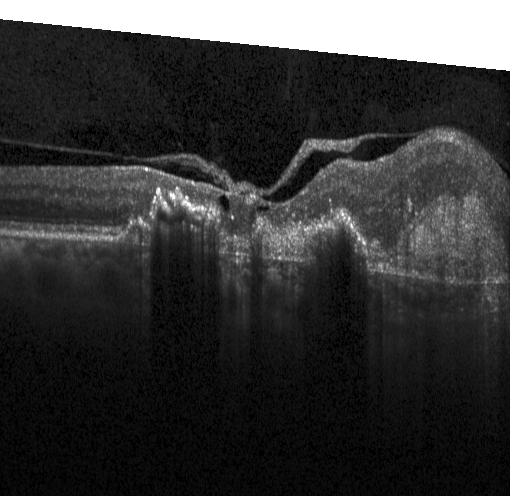
Retinal OCT B-scan. Spectral-domain optical coherence tomography
The scan shows choroidal neovascularization (CNV).